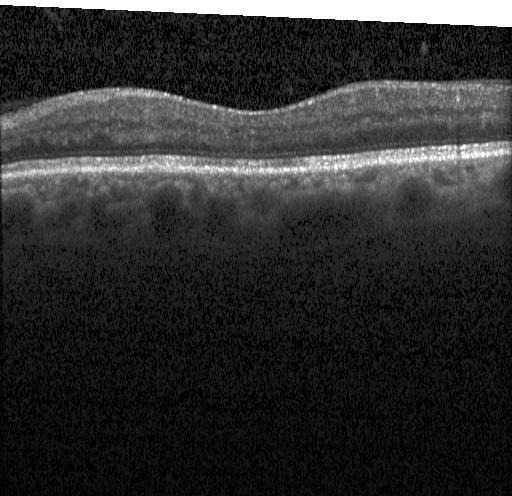
No choroidal neovascularization, diabetic macular edema, or drusen.